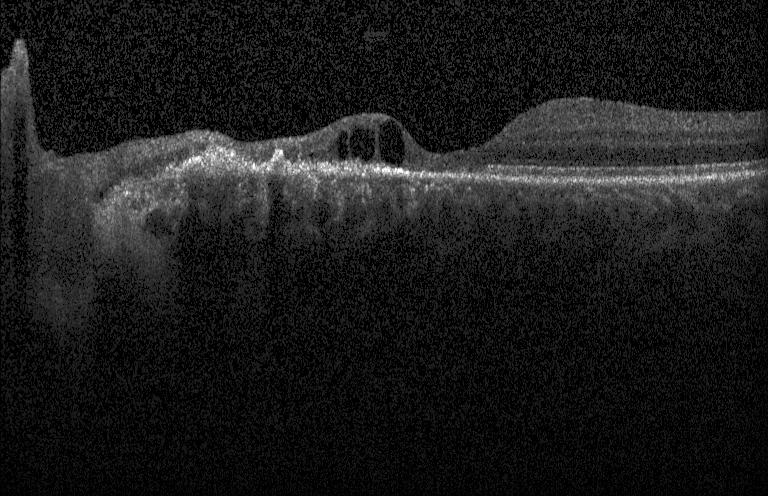 OCT scan showing a choroidal neovascular membrane.